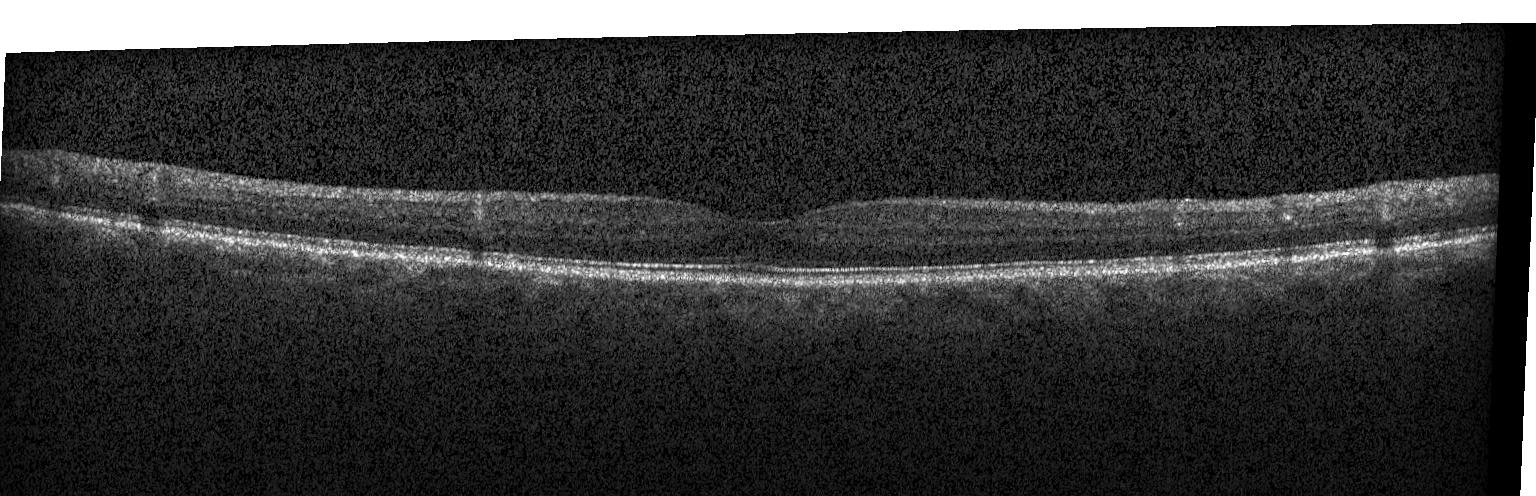
Diagnosis: no CNV, no DME, and no drusen.